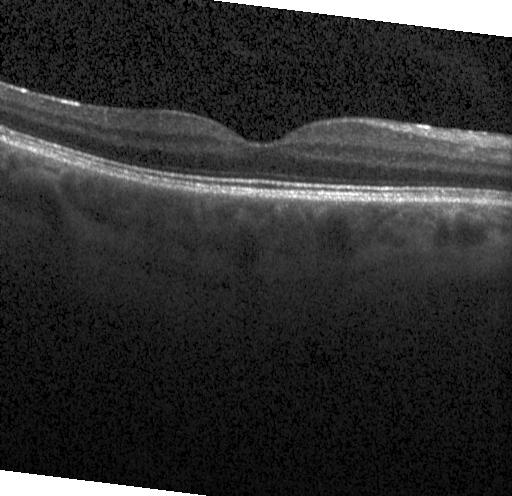 Optical coherence tomography B-scan, spectral-domain optical coherence tomography
Finding: no CNV, DME, or drusen.